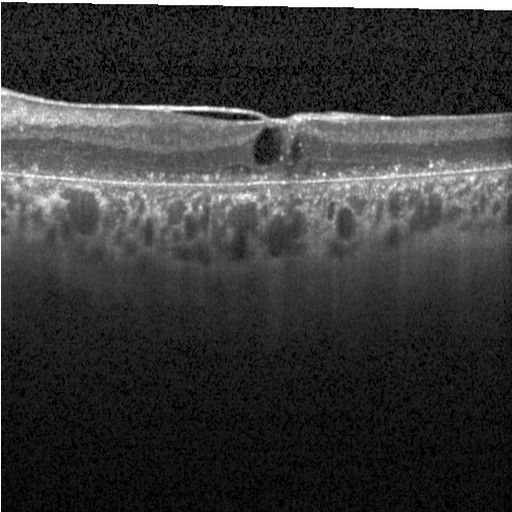

Diabetic macular edema (DME).